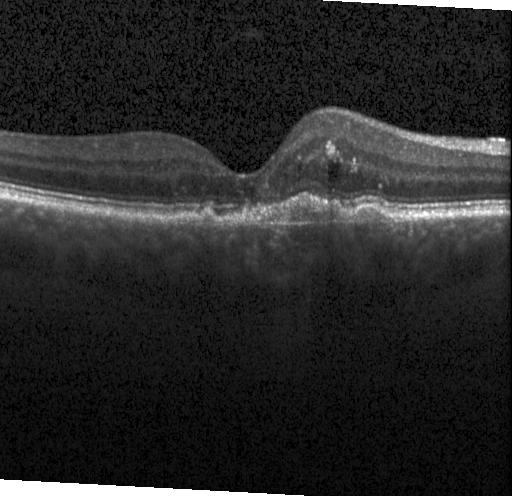 Spectral-domain optical coherence tomography, OCT B-scan — Impression: a choroidal neovascular membrane.